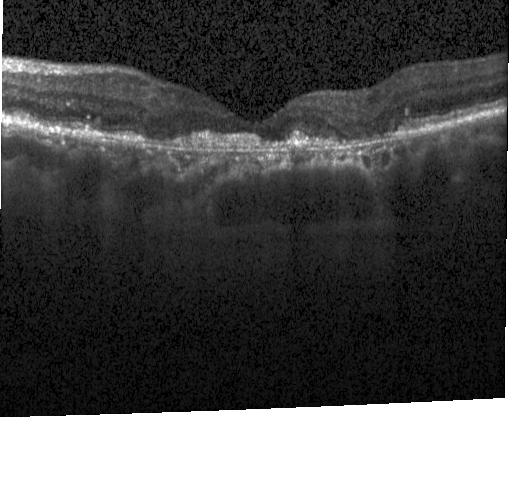

Macular OCT demonstrating CNV.